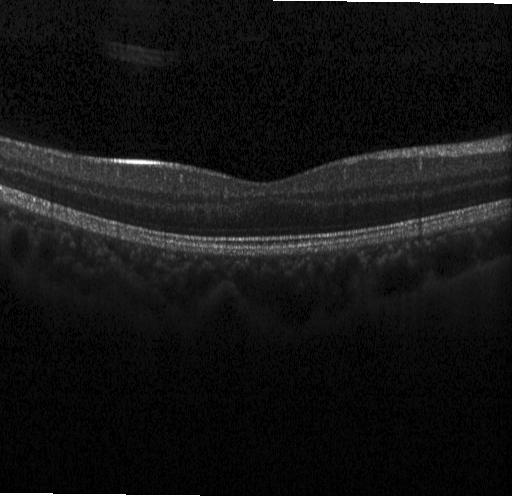
SD-OCT; optical coherence tomography scan
Finding: no choroidal neovascularization, diabetic macular edema, or drusen.